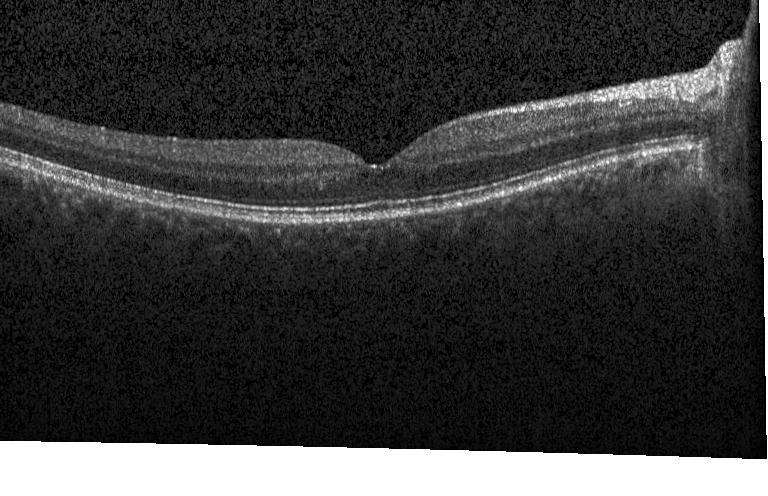 Macular OCT: no choroidal neovascularization, no diabetic macular edema, and no drusen.